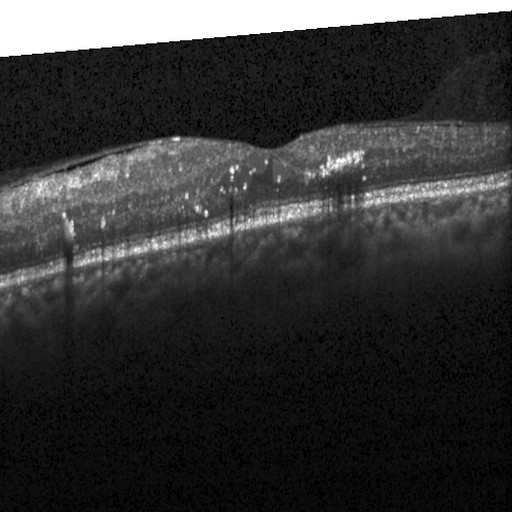

Retinal OCT cross-section; spectral-domain optical coherence tomography; fovea-centered
Diagnosis: diabetic macular edema (DME).